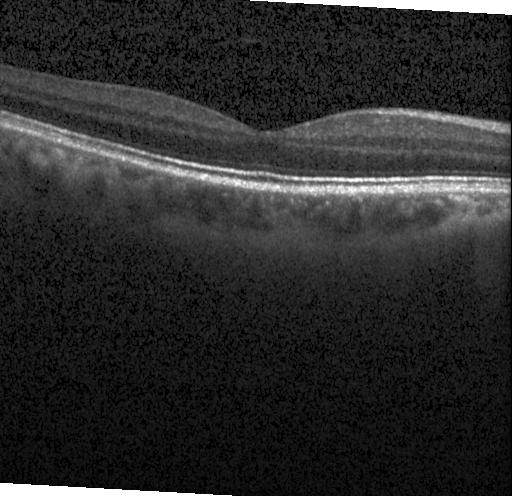

Optical coherence tomography B-scan · Heidelberg Spectralis.
Finding: neither CNV, DME, nor drusen.